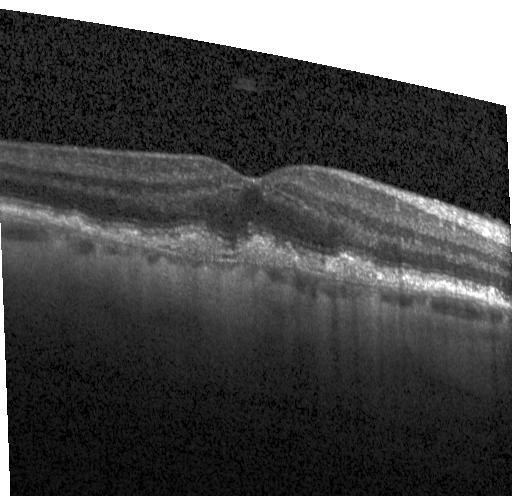
Dx: choroidal neovascularization (CNV).